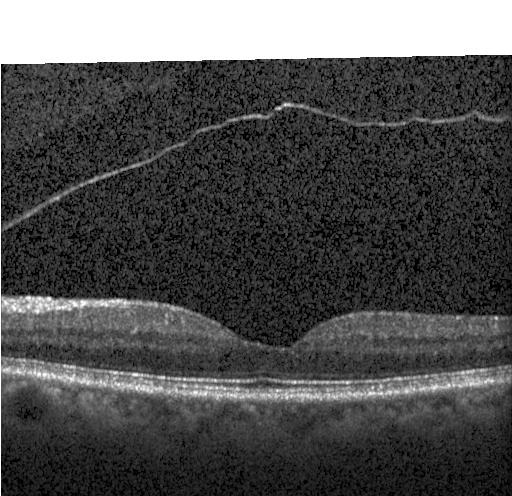
Heidelberg Spectralis OCT system. Spectral-domain OCT. Retinal OCT B-scan
Dx: no evidence of choroidal neovascularization, diabetic macular edema, or drusen.